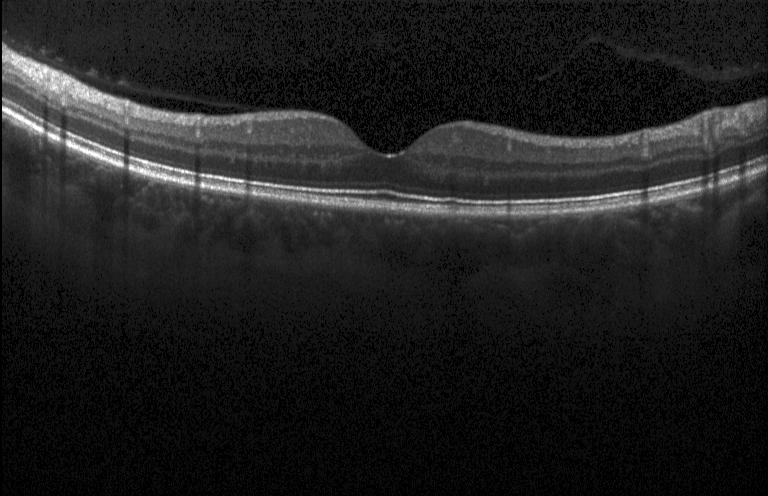
Spectral-domain optical coherence tomography, acquired on a Heidelberg Spectralis, horizontal scan through the fovea, retinal OCT B-scan — Dx: no choroidal neovascularization, no diabetic macular edema, and no drusen.